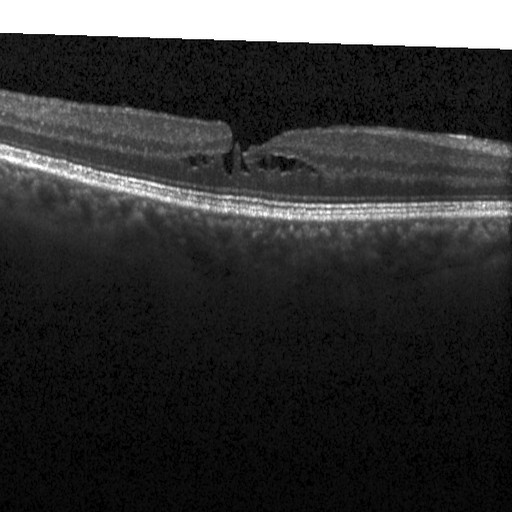 Diagnosis: diabetic macular edema (DME).